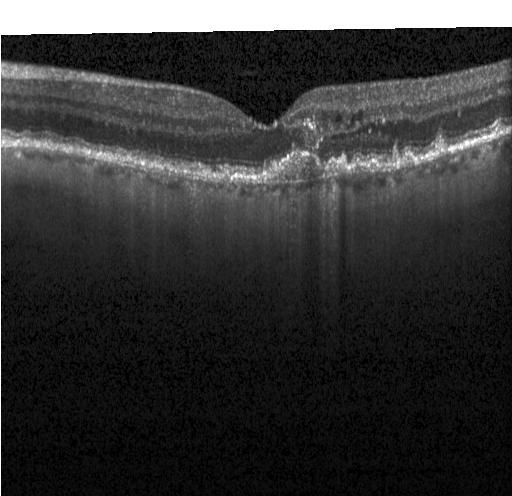

Retinal OCT cross-section; Heidelberg Spectralis; spectral-domain OCT; centered on the fovea. Dx: choroidal neovascularization (CNV).